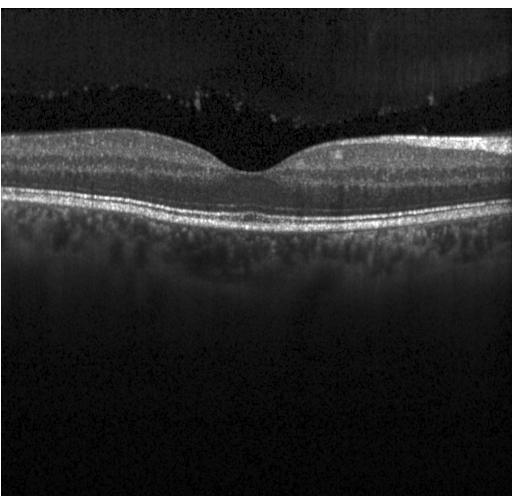

Impression: no evidence of choroidal neovascularization, diabetic macular edema, or drusen.